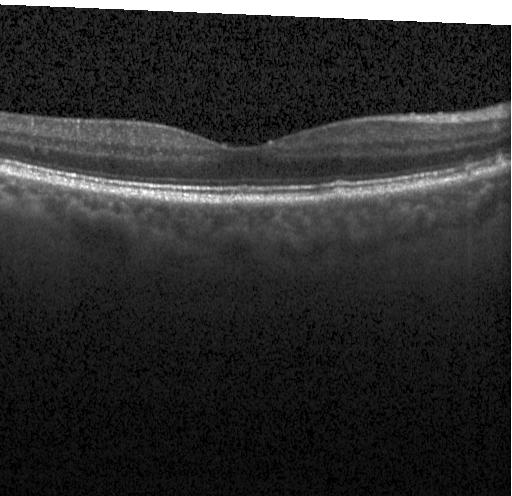
Retinal OCT B-scan. Spectral-domain OCT
Finding: no evidence of CNV, DME, or drusen.